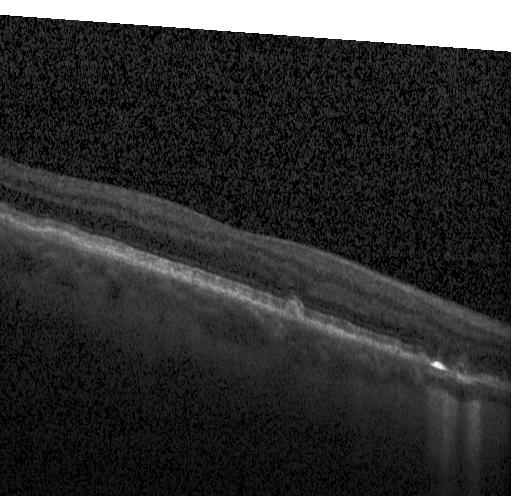
OCT finding: drusen.